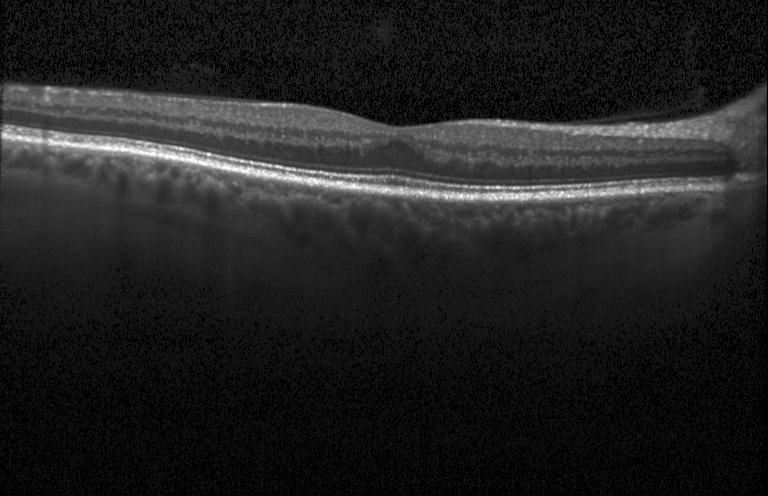

Optical coherence tomography B-scan, centered on the fovea, instrument: Heidelberg Spectralis
Dx: neither choroidal neovascularization, diabetic macular edema, nor drusen.